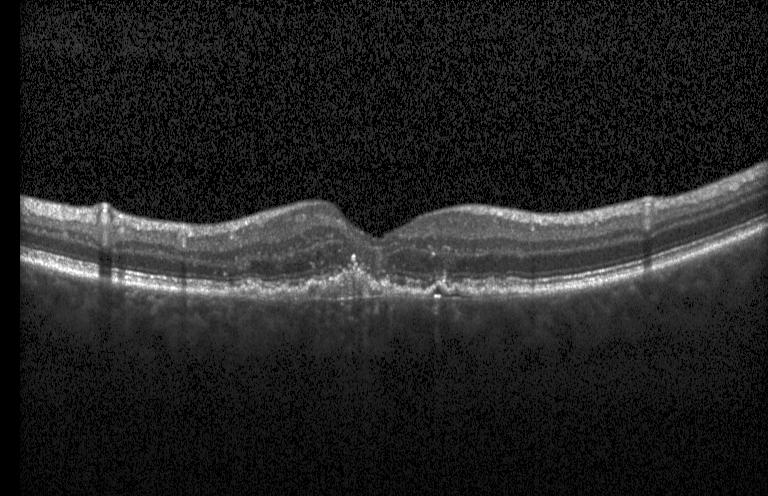
Acquired on a Heidelberg Spectralis. Optical coherence tomography scan. Spectral-domain OCT — Macular OCT: choroidal neovascularization (CNV).